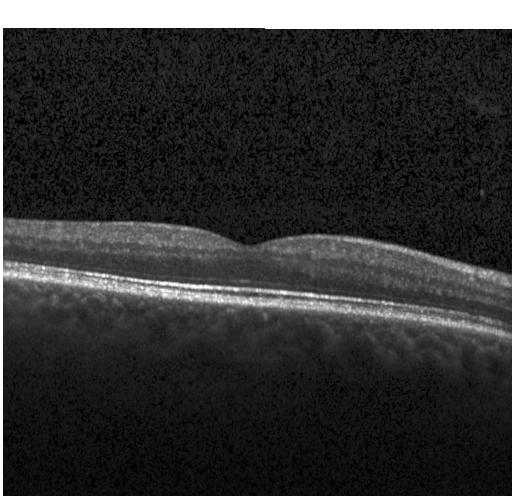 OCT B-scan, fovea-centered, SD-OCT
Finding: neither choroidal neovascularization, diabetic macular edema, nor drusen.